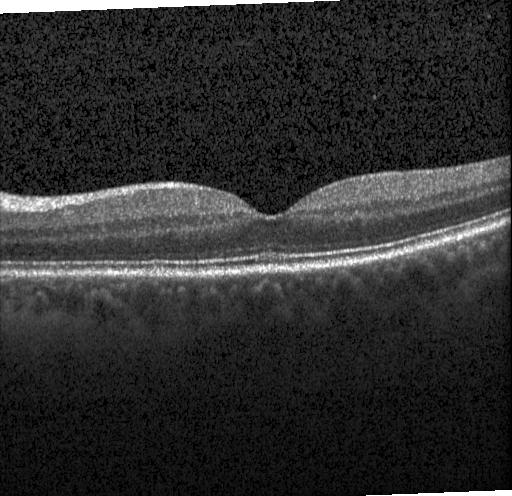 Retinal OCT cross-section · through the macula · Heidelberg Spectralis · SD-OCT.
Assessment: neither CNV, DME, nor drusen.